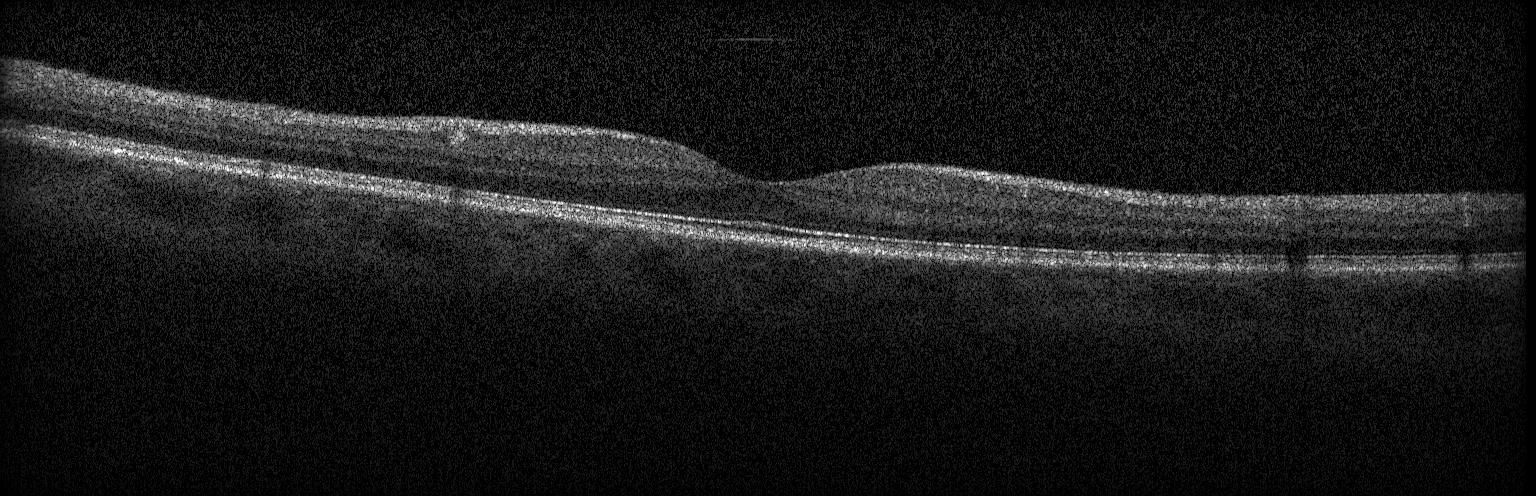

Retinal OCT B-scan · acquired on a Heidelberg Spectralis · horizontal scan through the fovea.
OCT finding: no evidence of CNV, DME, or drusen.